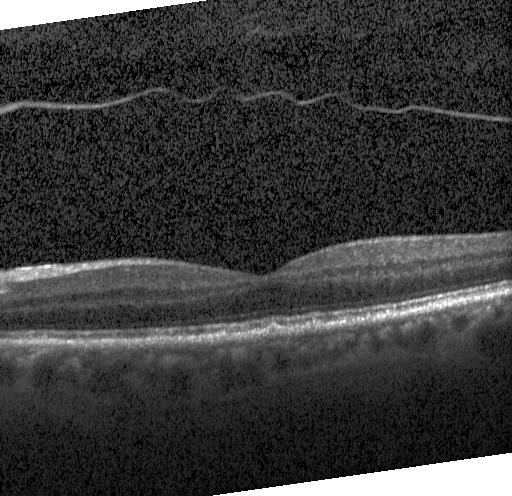

This B-scan demonstrates multiple drusen.